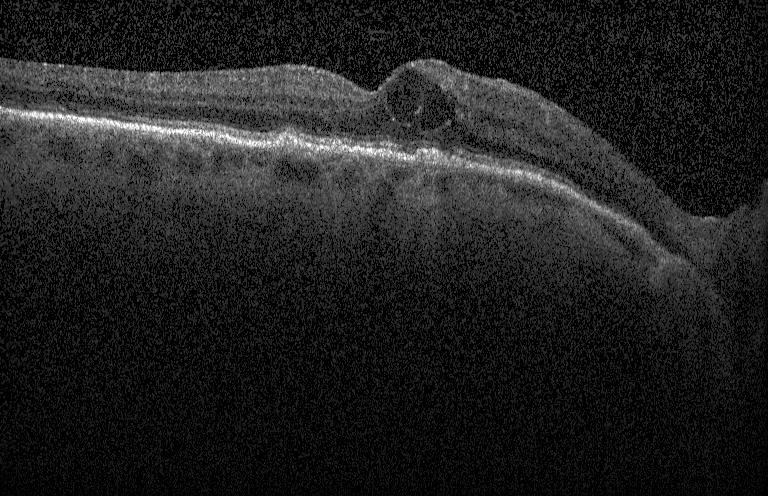
Diagnosis: a choroidal neovascular membrane.